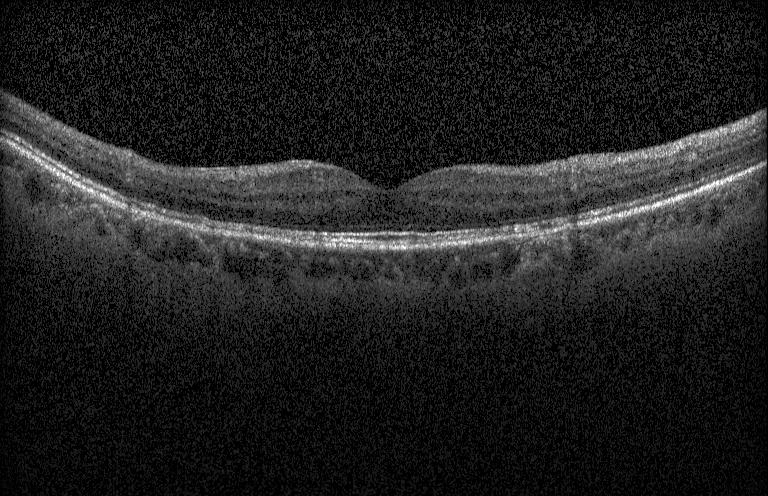
Heidelberg Spectralis, fovea-centered, retinal OCT cross-section. Impression: no choroidal neovascularization, diabetic macular edema, or drusen.